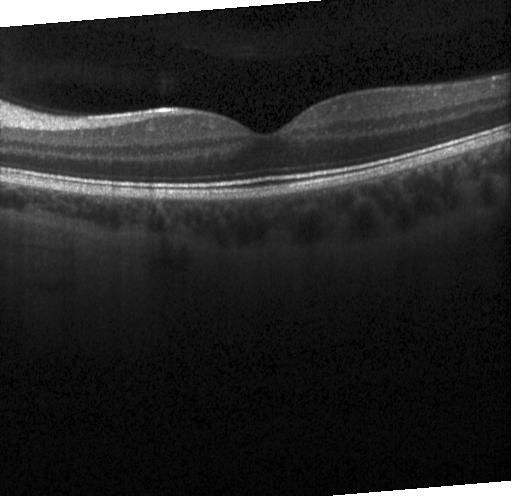 OCT B-scan showing no evidence of CNV, DME, or drusen.